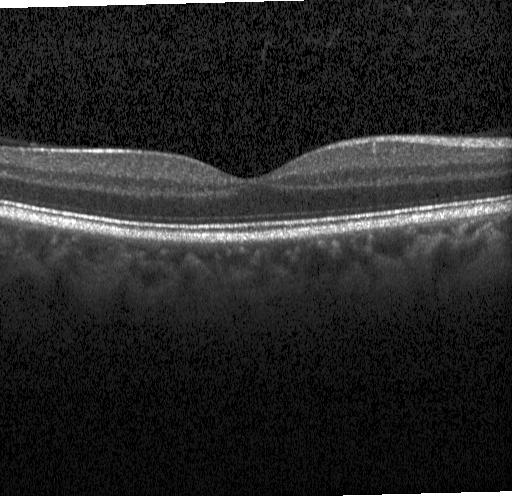
Spectral-domain optical coherence tomography. Retinal OCT B-scan. Centered on the fovea
Impression: neither CNV, DME, nor drusen.